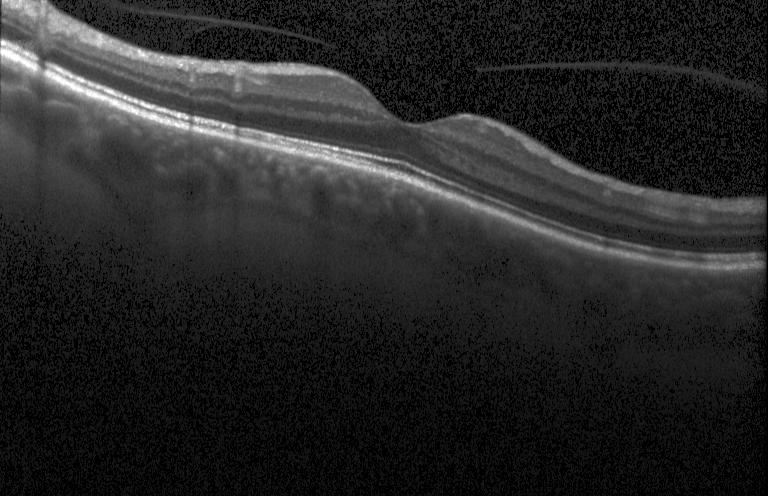

Diagnosis: no CNV, DME, or drusen.